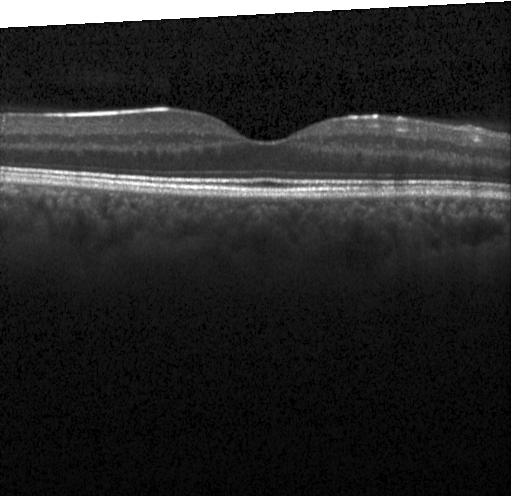 Spectral-domain OCT, retinal OCT B-scan.
Impression: neither choroidal neovascularization, diabetic macular edema, nor drusen.